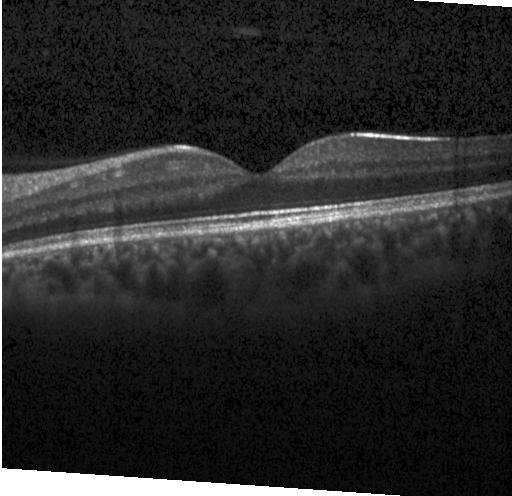

OCT B-scan
Dx: no choroidal neovascularization, diabetic macular edema, or drusen.